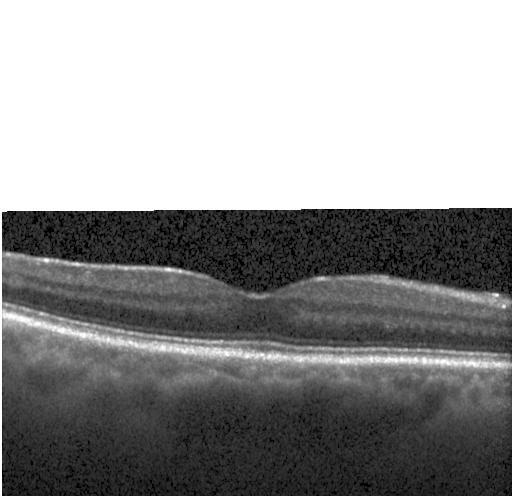
Centered on the fovea, Heidelberg Spectralis, SD-OCT, retinal OCT B-scan — OCT finding: no choroidal neovascularization, diabetic macular edema, or drusen.